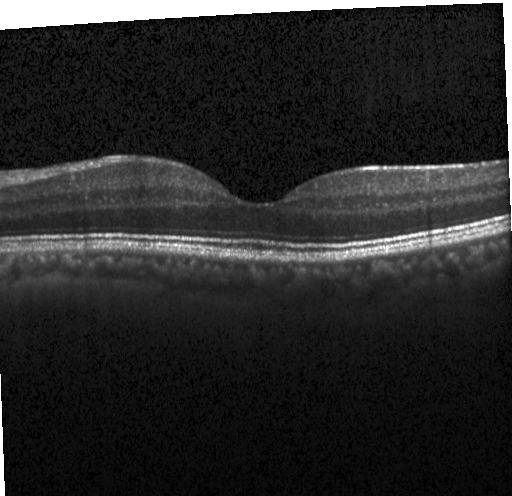

Impression: no evidence of choroidal neovascularization, diabetic macular edema, or drusen.